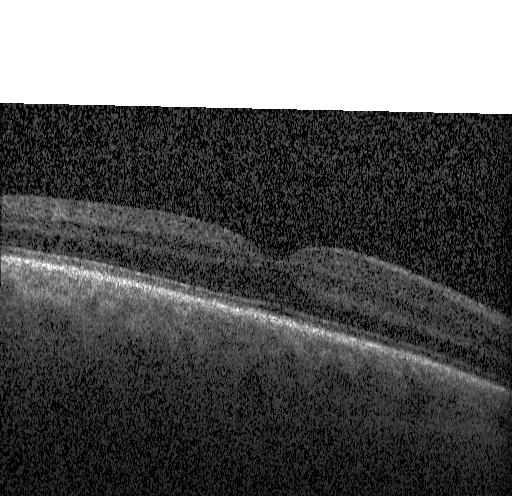

Optical coherence tomography B-scan, fovea-centered.
Diagnosis: no choroidal neovascularization, diabetic macular edema, or drusen.